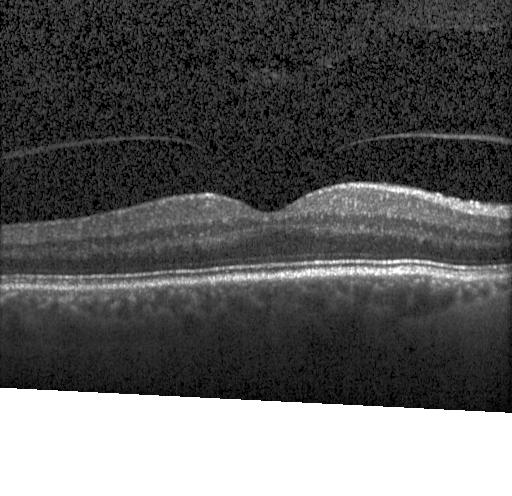
OCT scan showing no evidence of choroidal neovascularization, diabetic macular edema, or drusen.